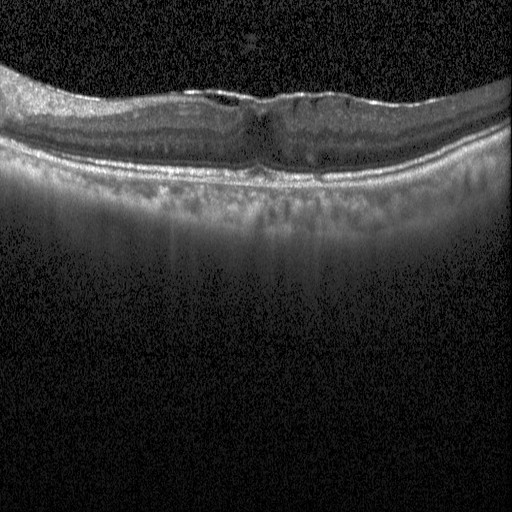

Retinal OCT cross-section; spectral-domain OCT; acquired on a Heidelberg Spectralis; horizontal scan through the fovea.
Finding: DME.